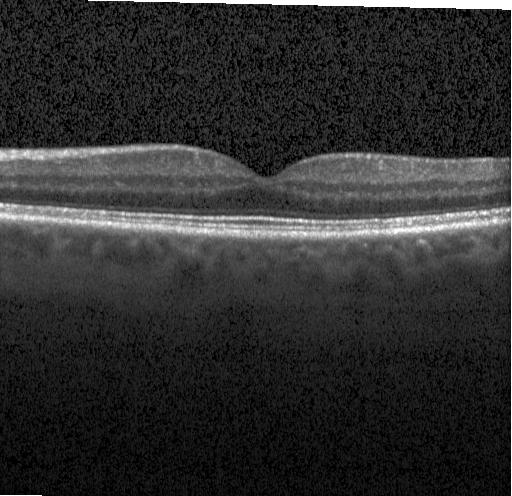

Spectral-domain optical coherence tomography; retinal OCT B-scan; instrument: Heidelberg Spectralis. Impression: no evidence of choroidal neovascularization, diabetic macular edema, or drusen.